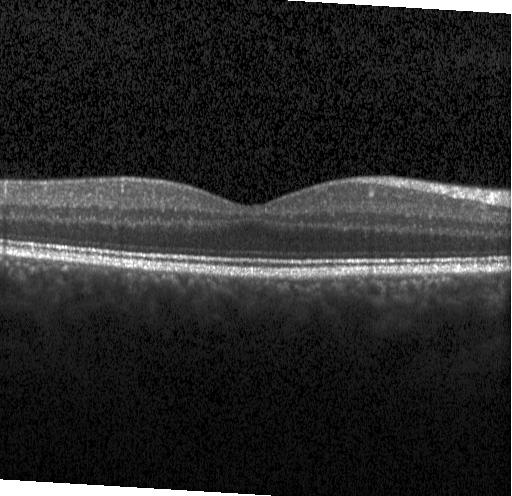

The scan shows no evidence of choroidal neovascularization, diabetic macular edema, or drusen.